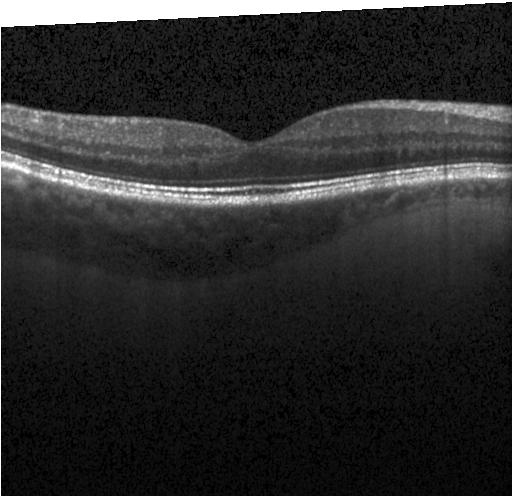 Retinal OCT cross-section.
Diagnosis: no choroidal neovascularization, diabetic macular edema, or drusen.